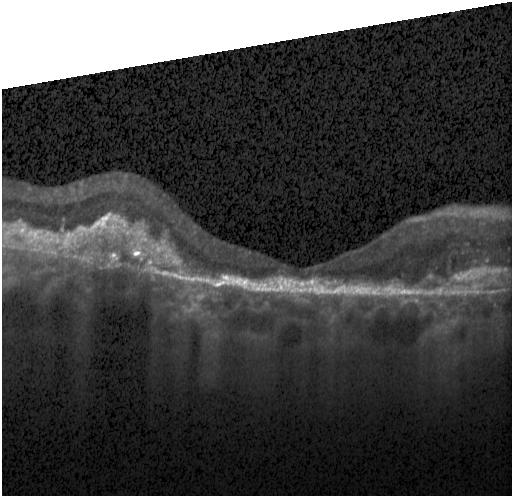
Heidelberg Spectralis OCT system. SD-OCT. OCT line scan. Centered on the fovea.
Finding: a choroidal neovascular membrane.